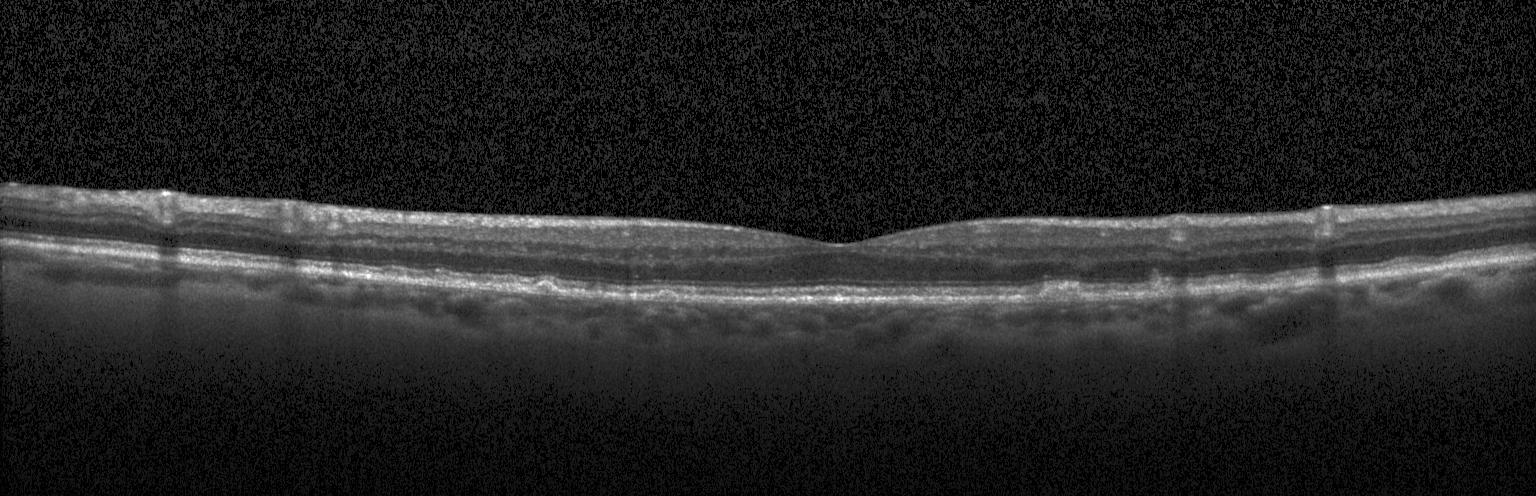
OCT B-scan.
Finding: multiple drusen.